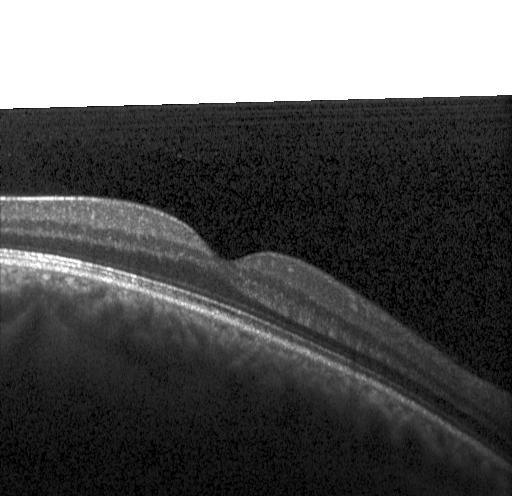

OCT B-scan. Impression: neither choroidal neovascularization, diabetic macular edema, nor drusen.